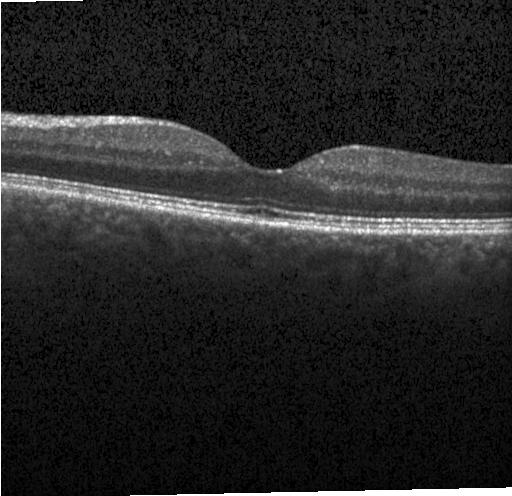 Impression: neither choroidal neovascularization, diabetic macular edema, nor drusen.